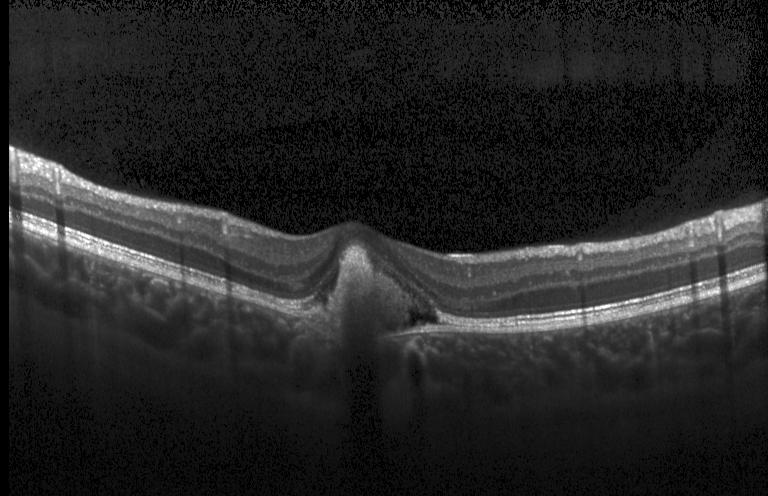
Macular OCT: choroidal neovascularization (CNV).